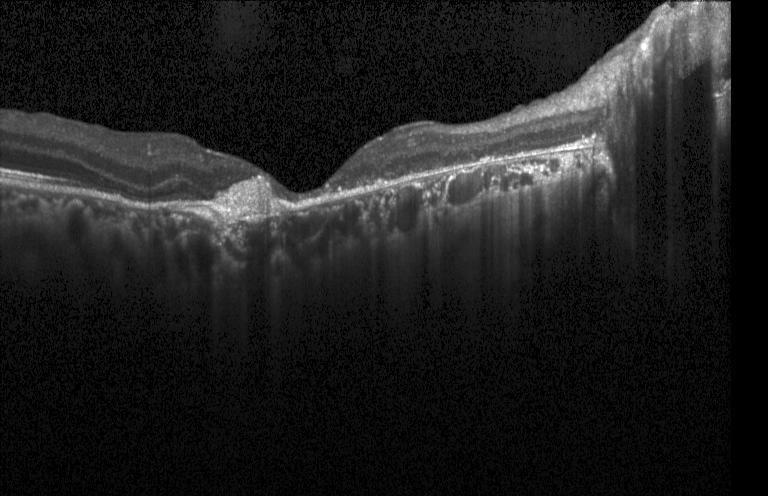
OCT B-scan. Instrument: Heidelberg Spectralis. Spectral-domain optical coherence tomography. Fovea-centered. Dx: CNV.